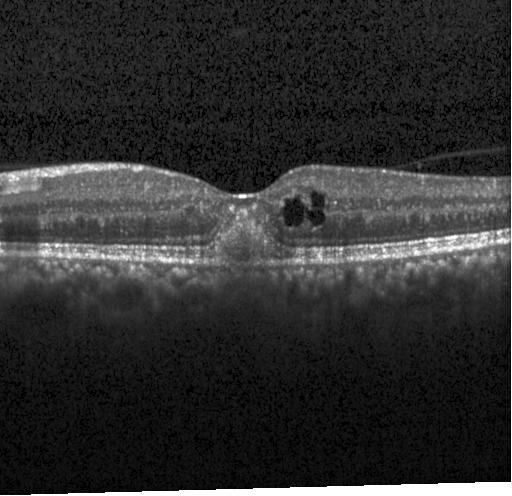

SD-OCT, retinal OCT cross-section. A choroidal neovascular membrane.